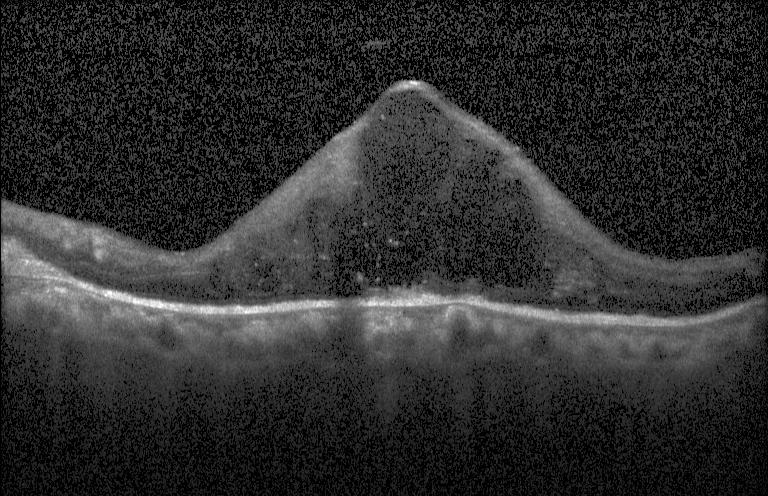

Retinal OCT cross-section showing diabetic macular edema.